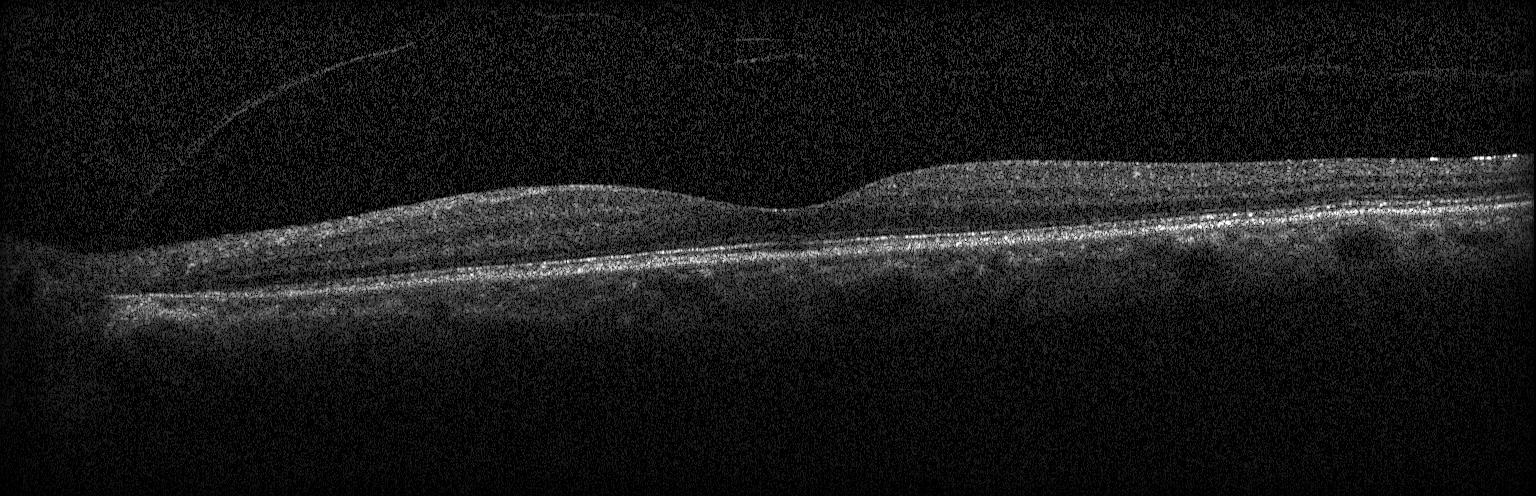 Retinal OCT B-scan — Assessment: neither choroidal neovascularization, diabetic macular edema, nor drusen.